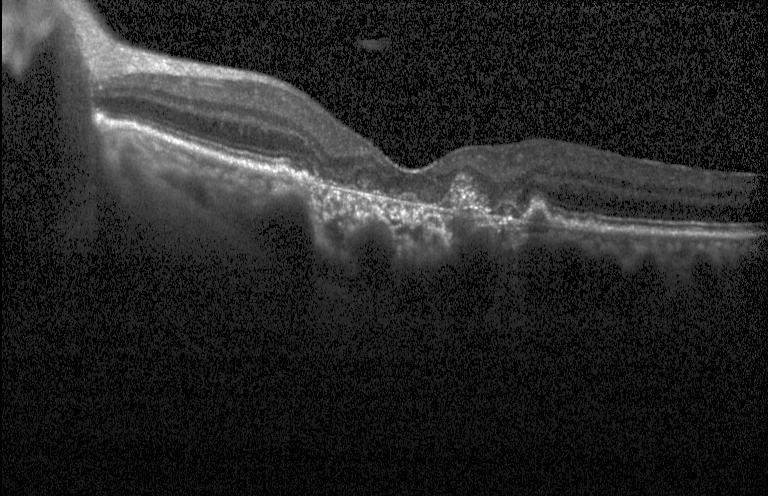

Diagnosis: a choroidal neovascular membrane.